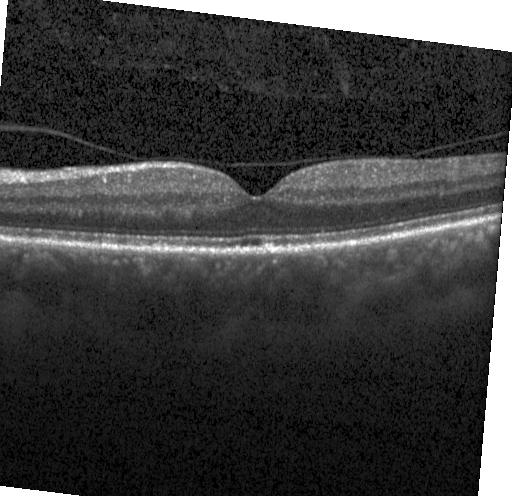
Heidelberg Spectralis OCT system; SD-OCT; horizontal scan through the fovea; retinal OCT cross-section. Diagnosis: neither choroidal neovascularization, diabetic macular edema, nor drusen.